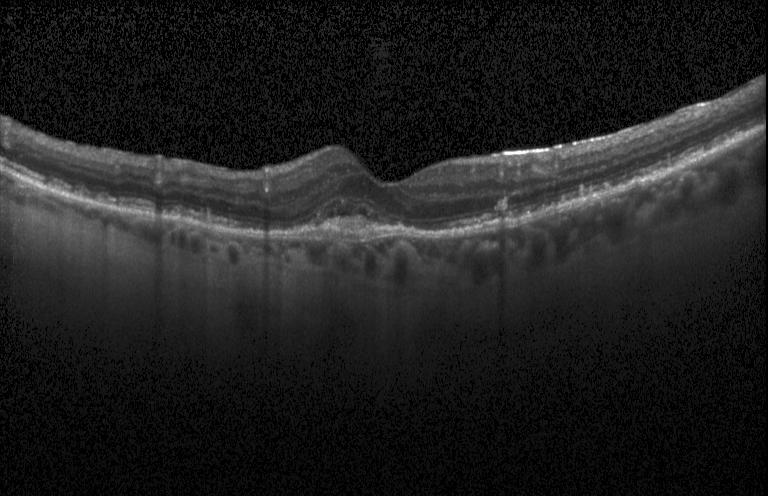
Through the macula. Spectral-domain OCT. OCT line scan
The scan shows a choroidal neovascular membrane.